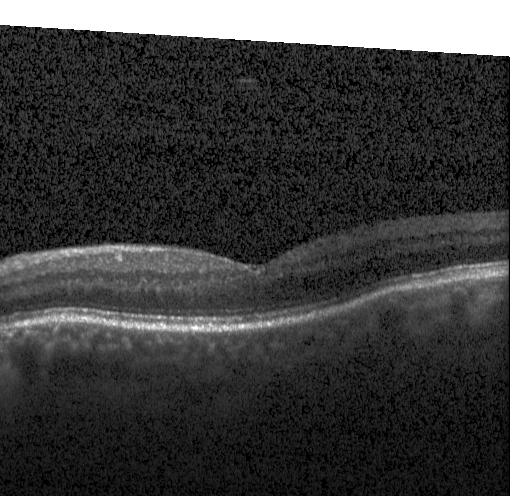
OCT finding: no CNV, no DME, and no drusen.